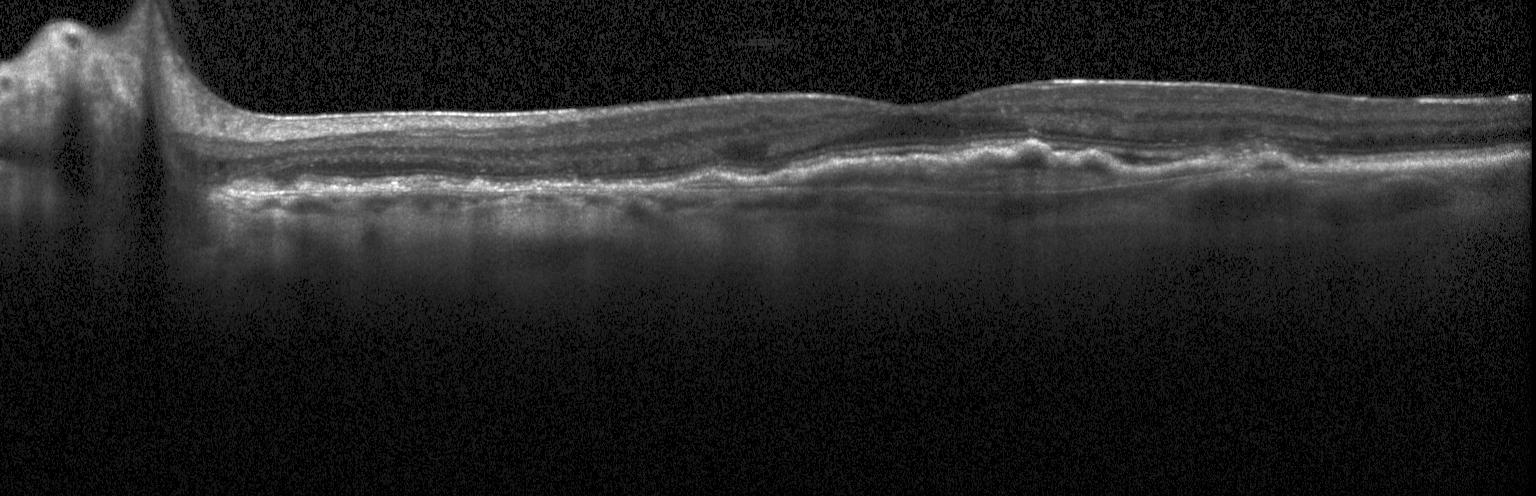 SD-OCT · optical coherence tomography B-scan — Finding: a choroidal neovascular membrane.